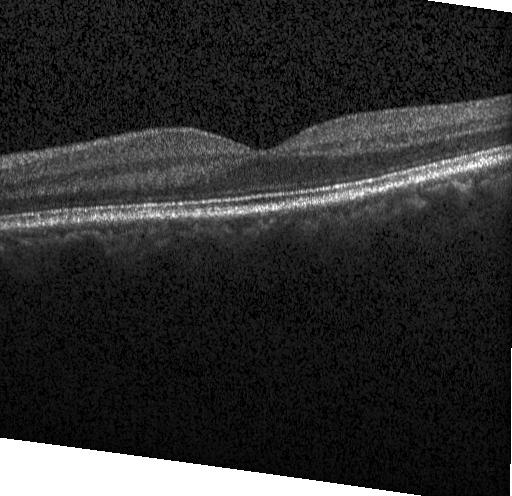

Macular OCT: no choroidal neovascularization, no diabetic macular edema, and no drusen.